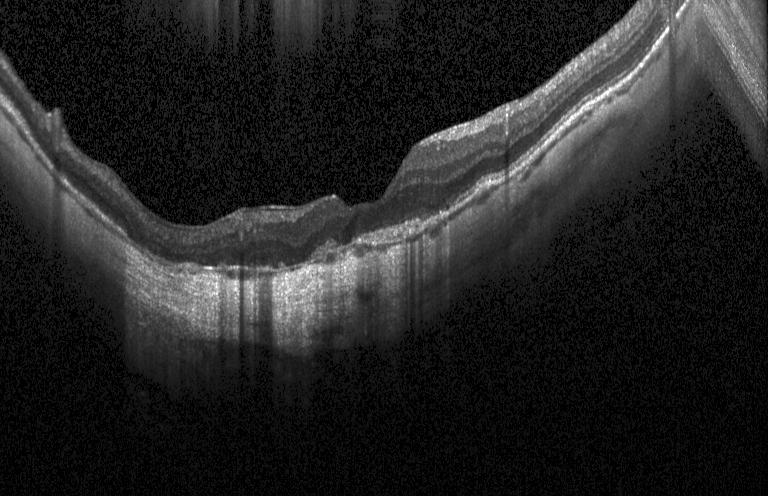

OCT B-scan. Macular scan. Spectral-domain OCT — This B-scan demonstrates a choroidal neovascular membrane.